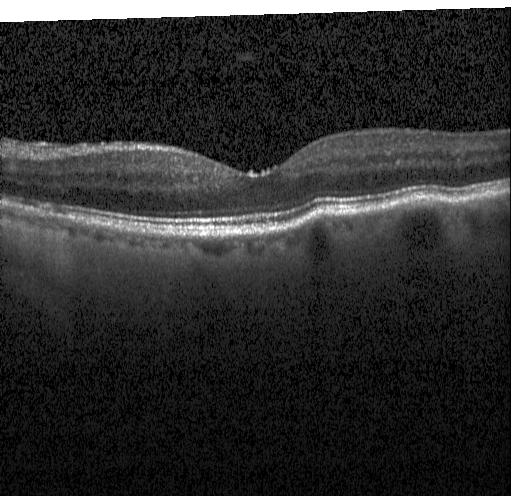
Diagnosis: sub-RPE drusenoid deposits.